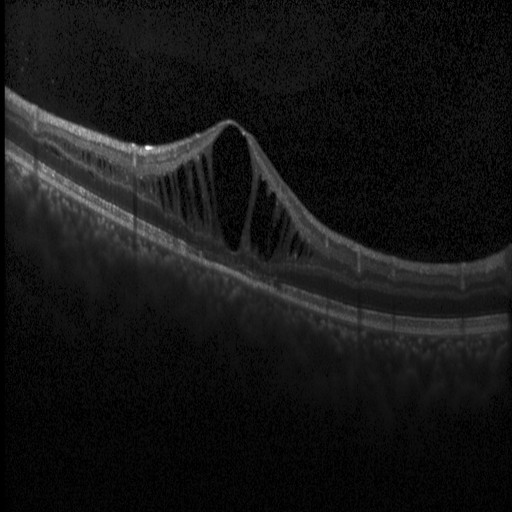

Retinal OCT B-scan — Assessment: DME.